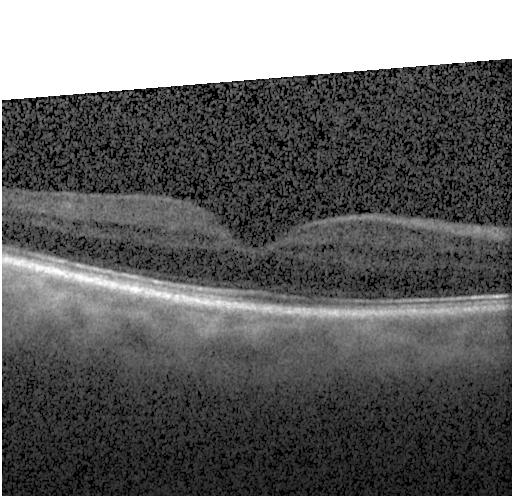 Heidelberg Spectralis, horizontal scan through the fovea, spectral-domain optical coherence tomography, retinal OCT cross-section.
Assessment: no CNV, DME, or drusen.